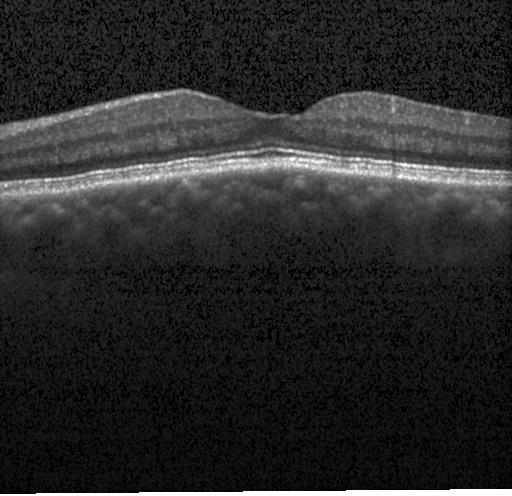 Optical coherence tomography B-scan; SD-OCT; Heidelberg Spectralis OCT system; centered on the fovea — Macular OCT: no evidence of choroidal neovascularization, diabetic macular edema, or drusen.